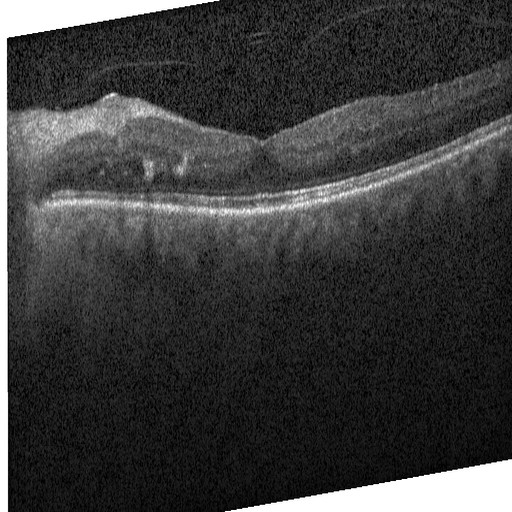 Macular OCT: diabetic macular edema (DME).